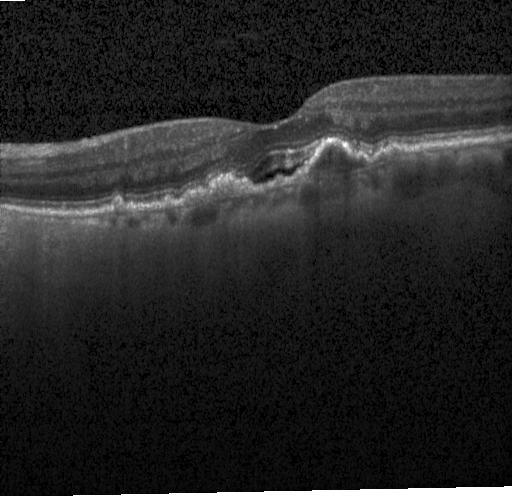

Finding: a choroidal neovascular membrane.